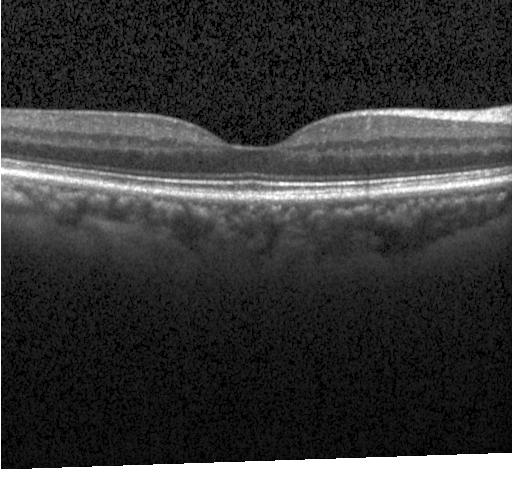

Finding: no choroidal neovascularization, diabetic macular edema, or drusen.